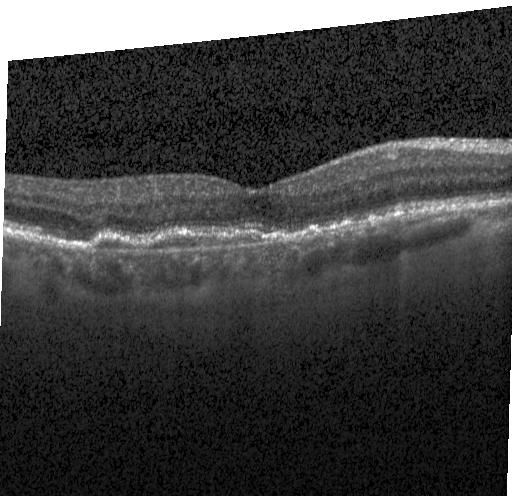
Heidelberg Spectralis, spectral-domain optical coherence tomography, centered on the fovea, OCT line scan.
This B-scan demonstrates choroidal neovascularization (CNV).